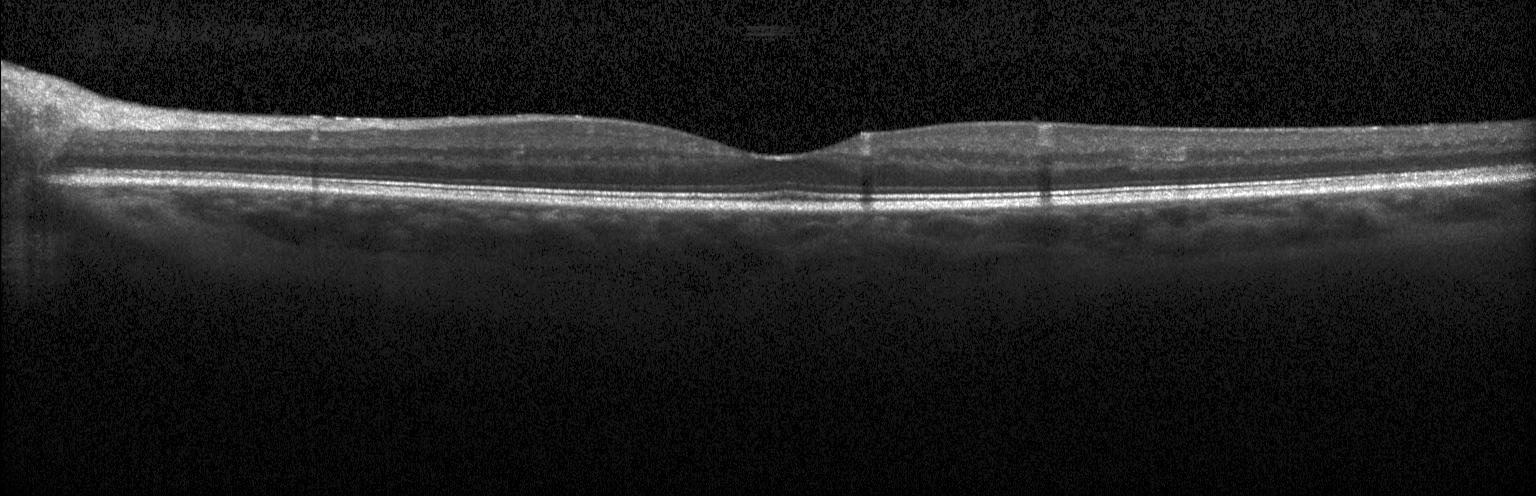
OCT B-scan. Heidelberg Spectralis
Finding: no evidence of choroidal neovascularization, diabetic macular edema, or drusen.